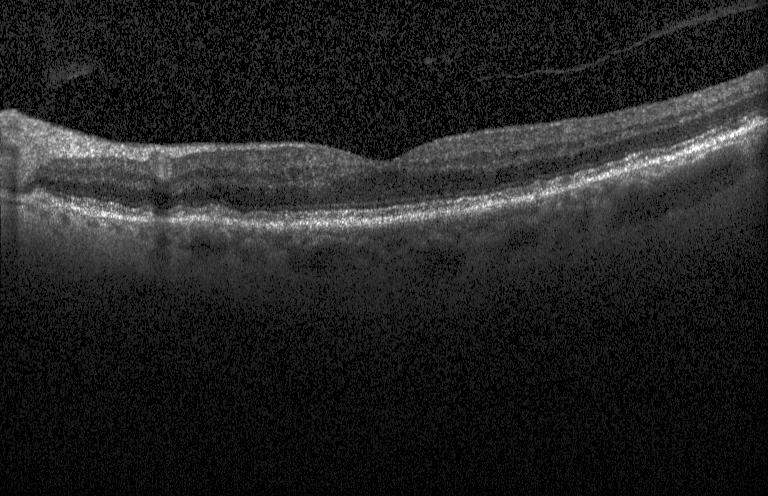 Heidelberg Spectralis · optical coherence tomography scan — Finding: drusen.